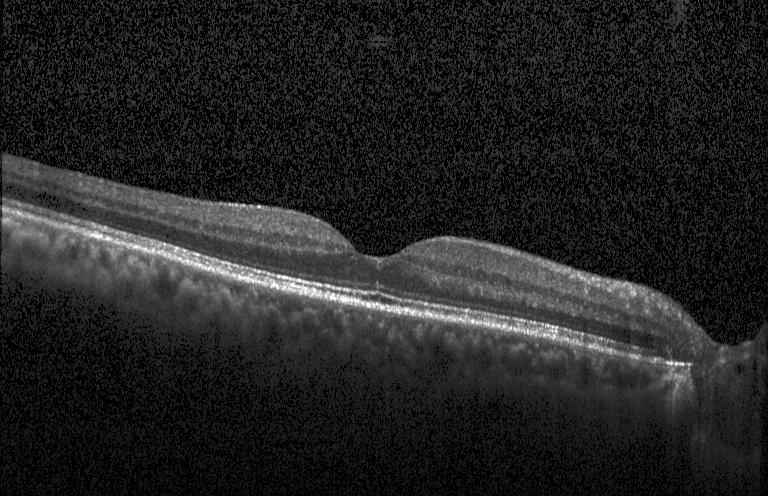

Spectral-domain OCT, fovea-centered, optical coherence tomography scan.
Assessment: no choroidal neovascularization, diabetic macular edema, or drusen.